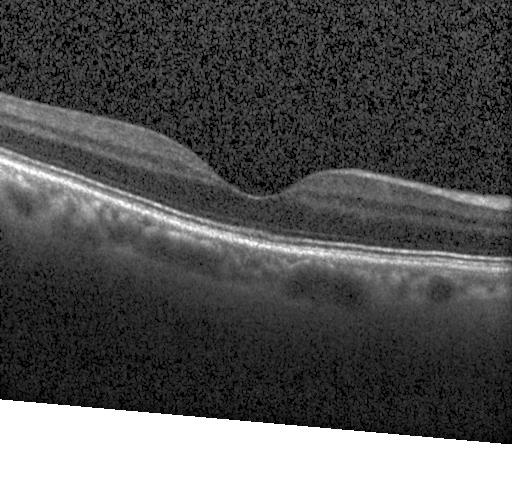
SD-OCT, fovea-centered, retinal OCT B-scan.
Diagnosis: no CNV, no DME, and no drusen.